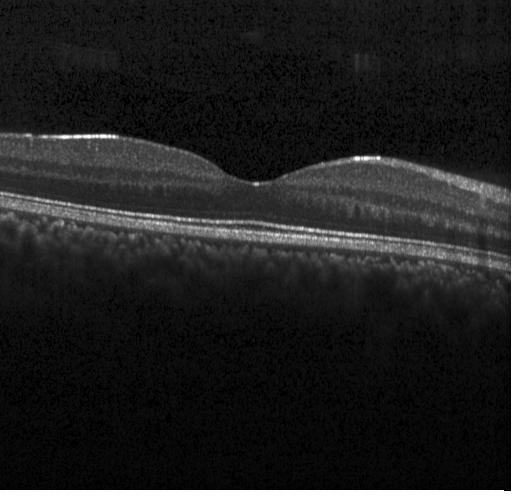 Macular OCT: no CNV, no DME, and no drusen.